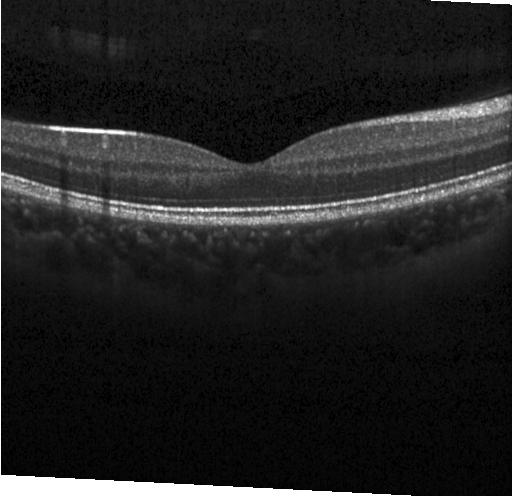 Retinal OCT cross-section, instrument: Heidelberg Spectralis, spectral-domain OCT — Impression: neither choroidal neovascularization, diabetic macular edema, nor drusen.